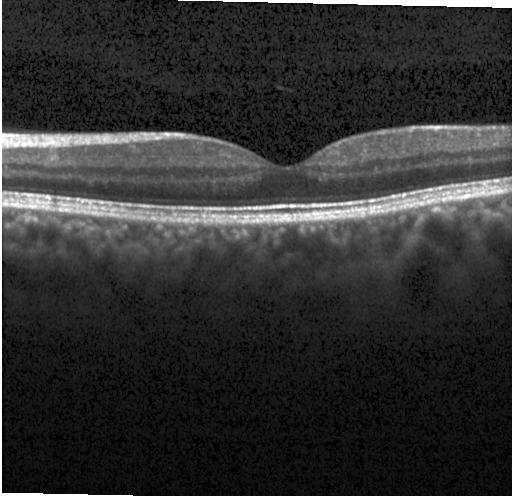
Heidelberg Spectralis, horizontal scan through the fovea, spectral-domain optical coherence tomography, optical coherence tomography B-scan — No CNV, DME, or drusen.